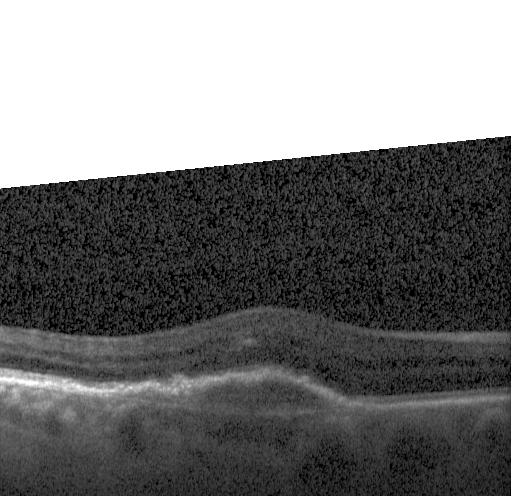

Macular OCT demonstrating a choroidal neovascular membrane.